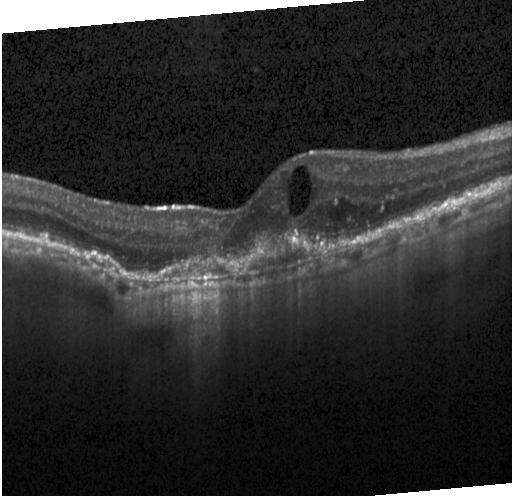 Heidelberg Spectralis OCT system · optical coherence tomography scan
Impression: a choroidal neovascular membrane.